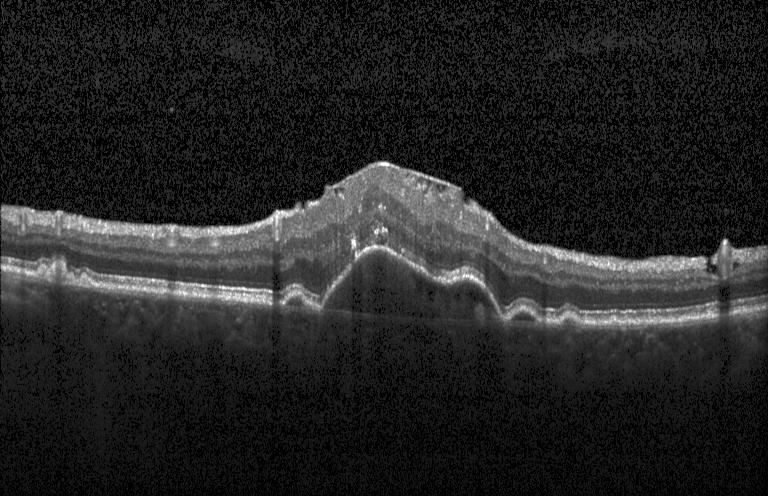 Retinal OCT cross-section, Heidelberg Spectralis, centered on the fovea.
Diagnosis: a choroidal neovascular membrane.